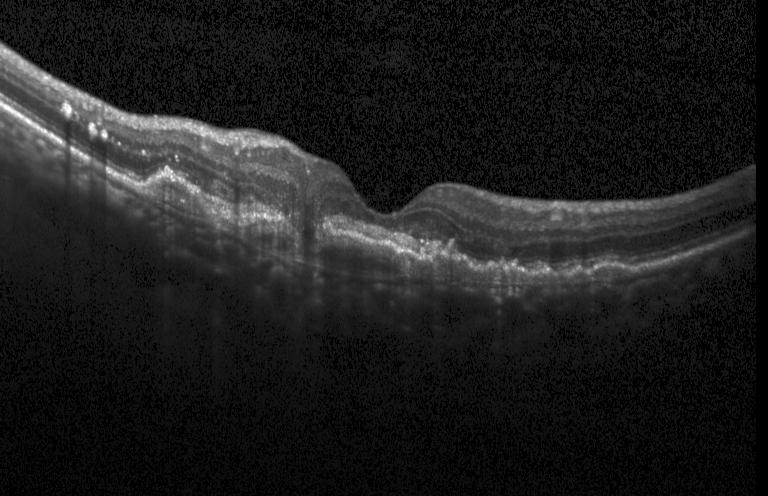
Heidelberg Spectralis, horizontal scan through the fovea, OCT B-scan — Dx: choroidal neovascularization (CNV).